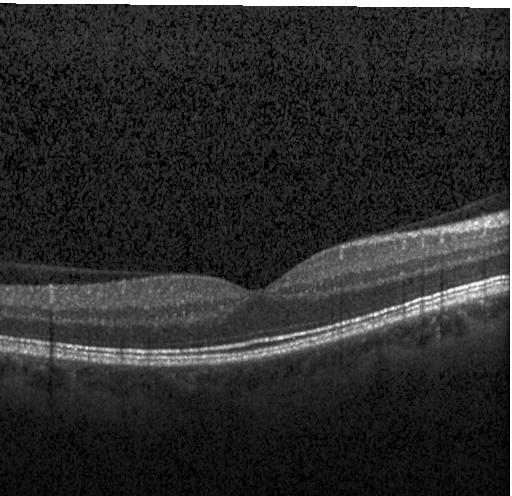
Retinal OCT cross-section. Spectral-domain OCT. Macular scan. OCT finding: no choroidal neovascularization, no diabetic macular edema, and no drusen.